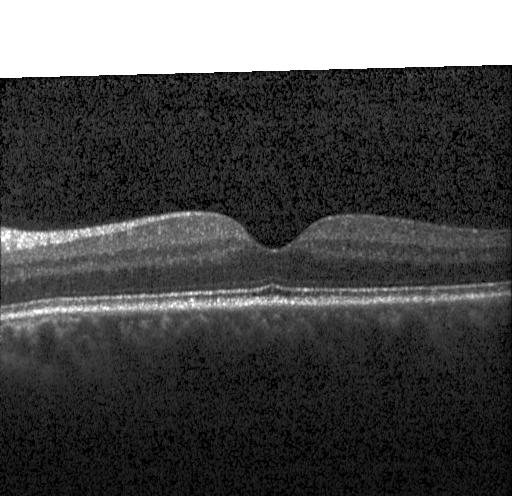
Finding: neither CNV, DME, nor drusen.